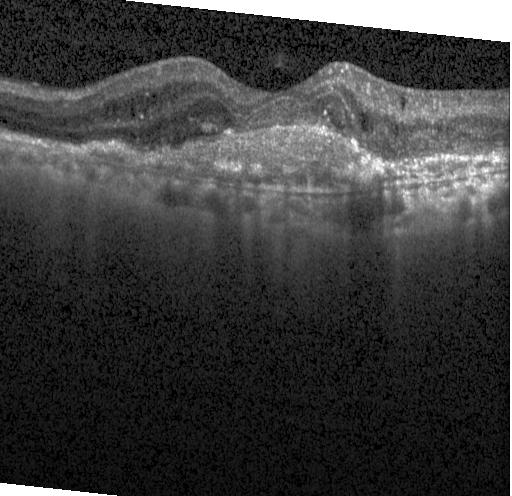 Spectral-domain optical coherence tomography · acquired on a Heidelberg Spectralis · retinal OCT B-scan · horizontal scan through the fovea.
Diagnosis: a choroidal neovascular membrane.